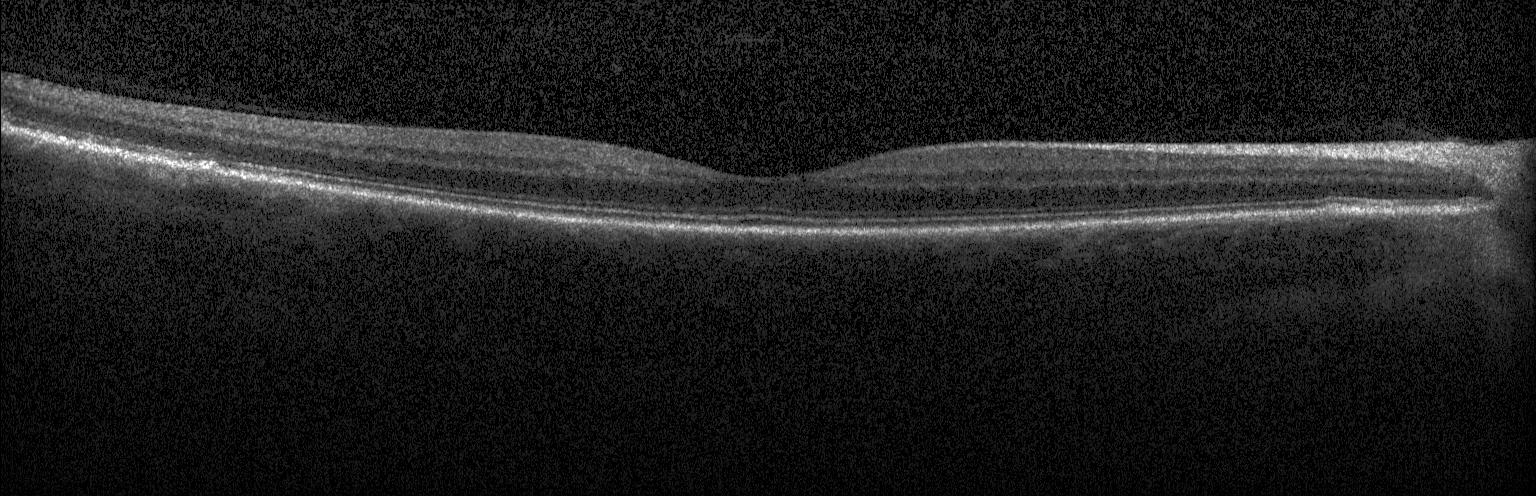 Retinal OCT B-scan. SD-OCT. Finding: no evidence of CNV, DME, or drusen.